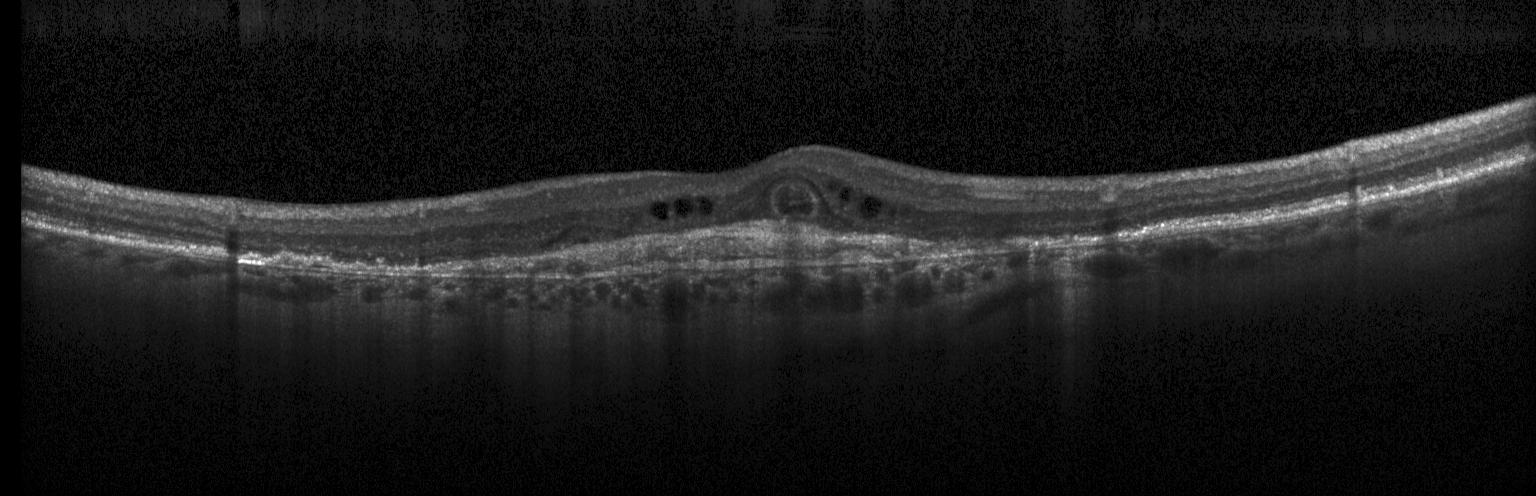

Finding: choroidal neovascularization (CNV).